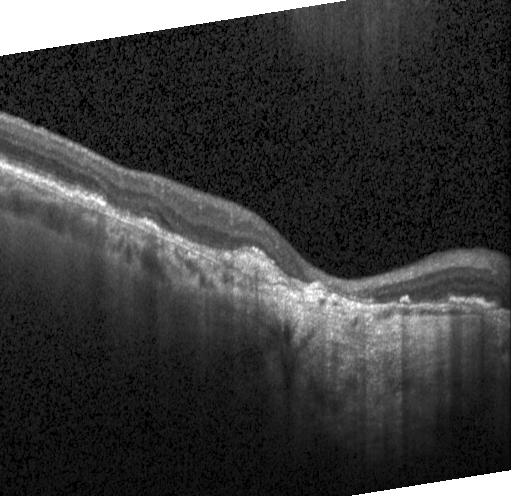
OCT B-scan. Heidelberg Spectralis OCT system. Macular scan. Assessment: choroidal neovascularization (CNV).